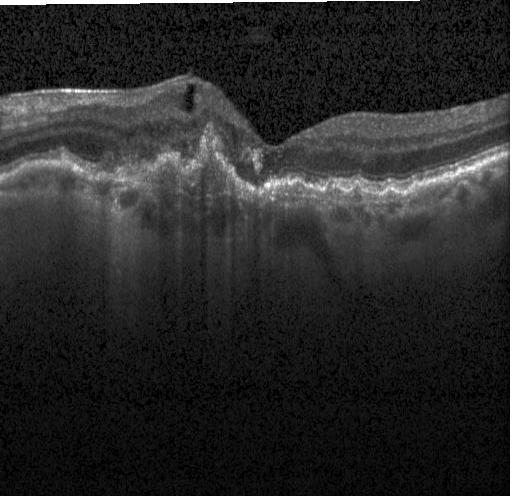 SD-OCT. Fovea-centered. Retinal OCT B-scan.
Finding: a choroidal neovascular membrane.